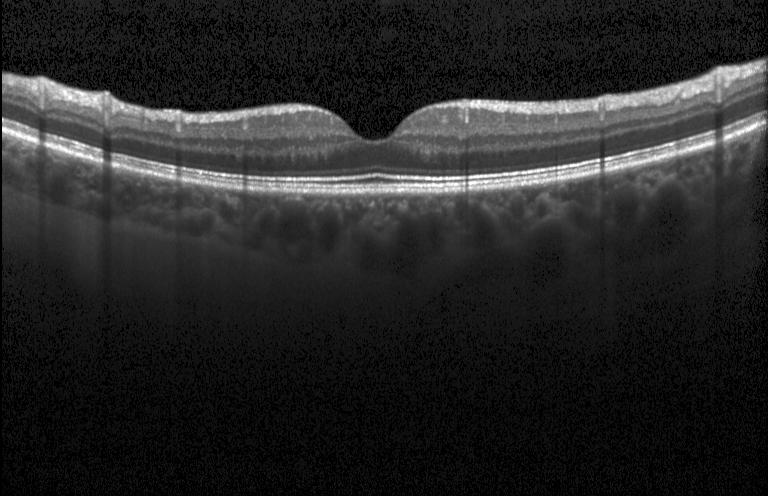

Impression: neither choroidal neovascularization, diabetic macular edema, nor drusen.